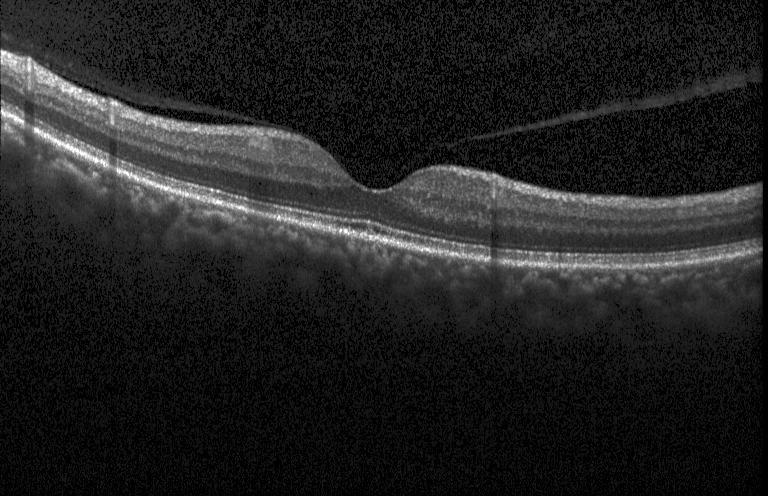

OCT line scan.
Diagnosis: no CNV, no DME, and no drusen.